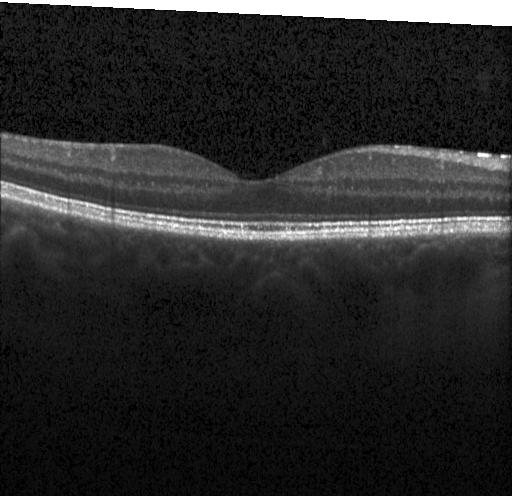
Through the macula. Spectral-domain OCT. Optical coherence tomography scan.
Diagnosis: no choroidal neovascularization, no diabetic macular edema, and no drusen.